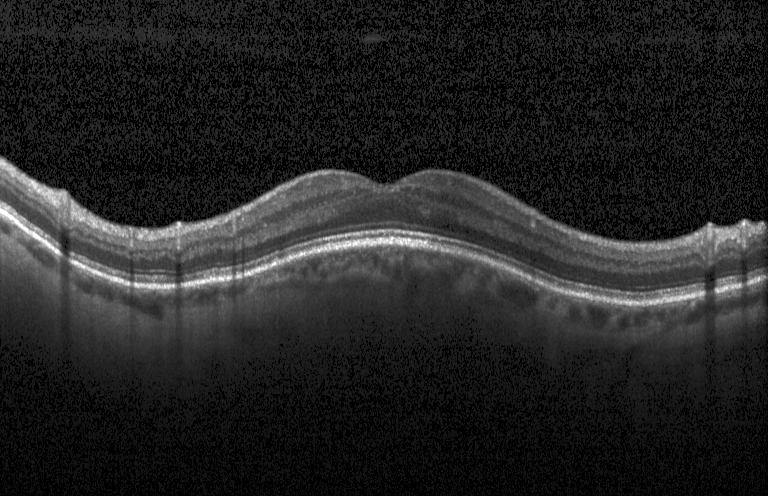

Retinal OCT B-scan
No CNV, DME, or drusen.